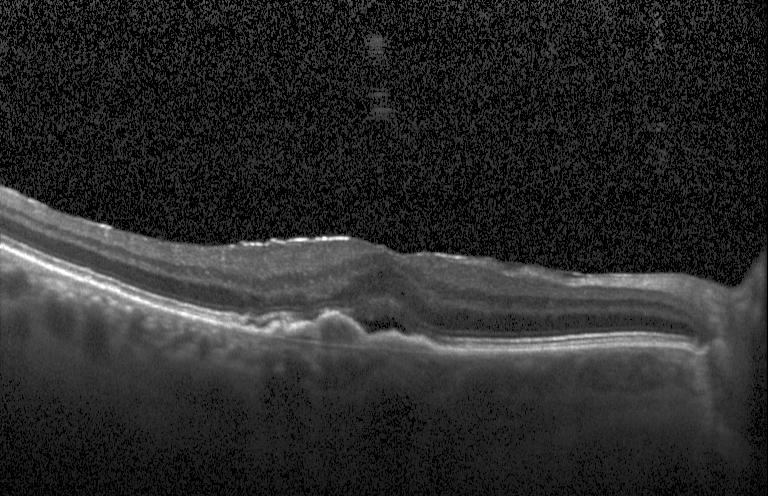
The scan shows a choroidal neovascular membrane.